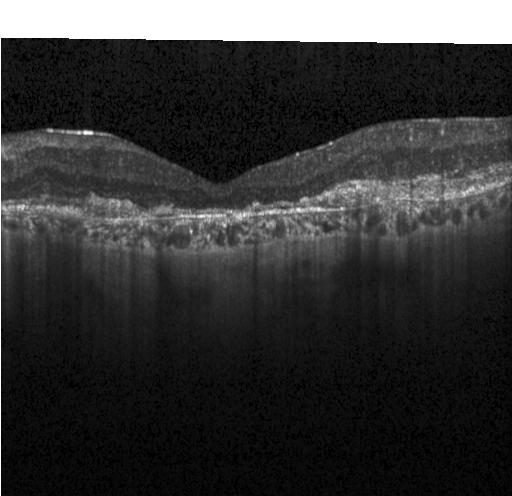

OCT line scan. Horizontal scan through the fovea.
Impression: choroidal neovascularization (CNV).